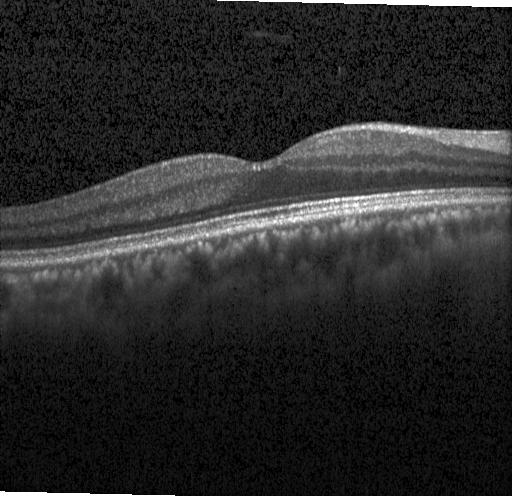 Finding: no evidence of CNV, DME, or drusen.